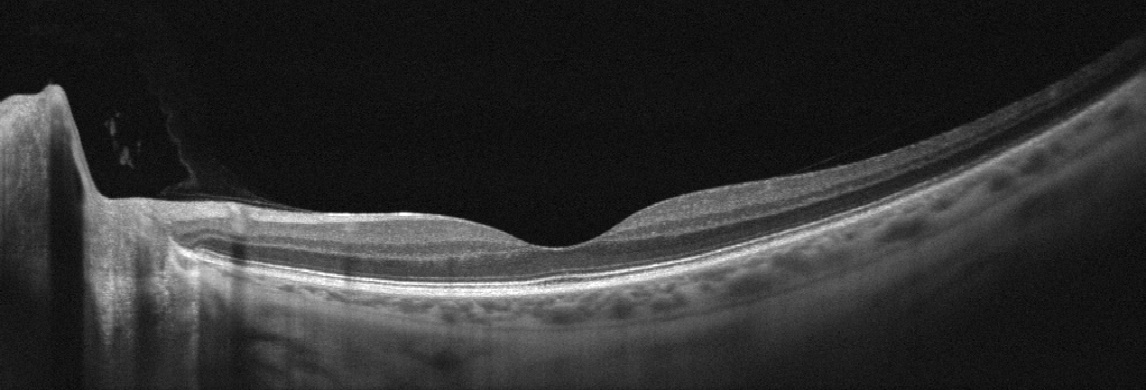 Macular OCT: absence of AMD, DME, ERM, RAO, RVO, and vitreomacular interface disease.